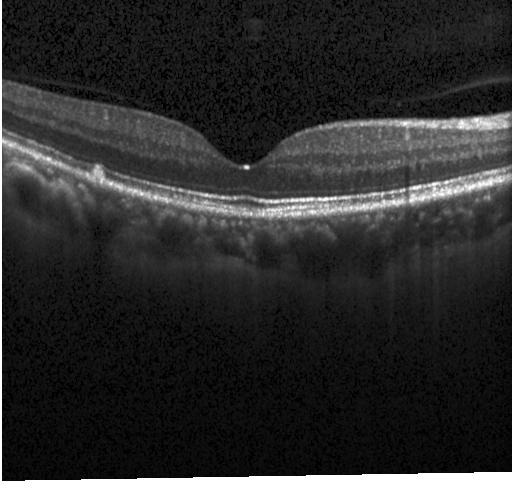
Assessment: multiple drusen.